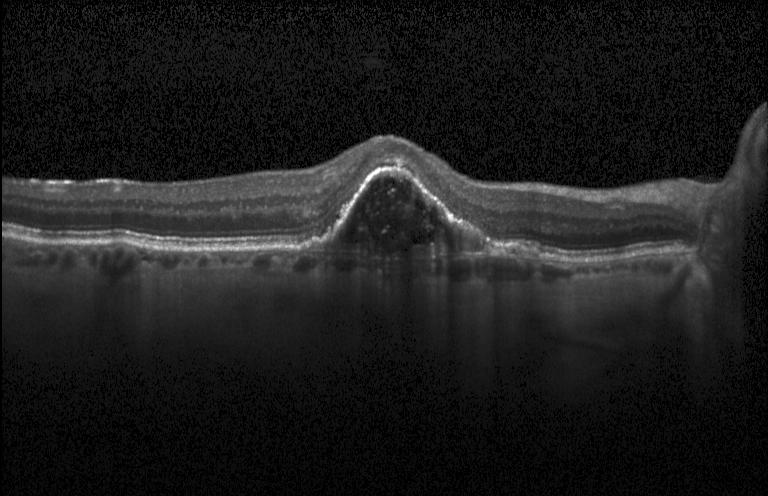
Optical coherence tomography scan. Spectral-domain optical coherence tomography. Through the macula. Acquired on a Heidelberg Spectralis.
Macular OCT: a choroidal neovascular membrane.